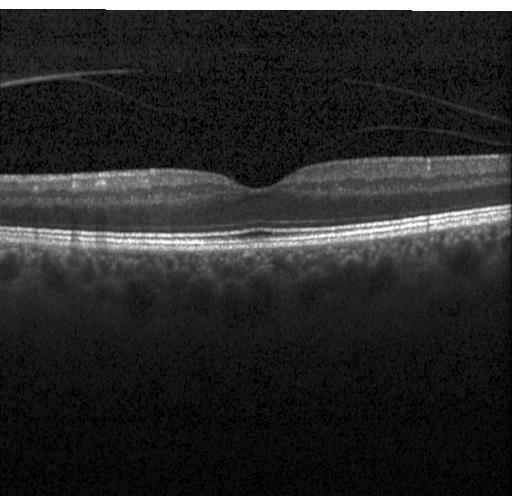

Macular scan. SD-OCT. Retinal OCT B-scan. Finding: neither choroidal neovascularization, diabetic macular edema, nor drusen.